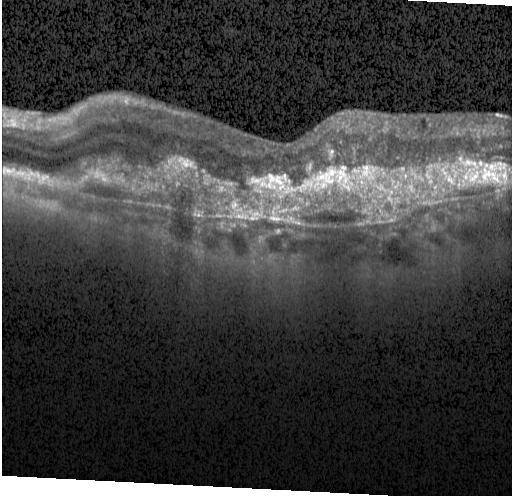 Impression: a choroidal neovascular membrane.